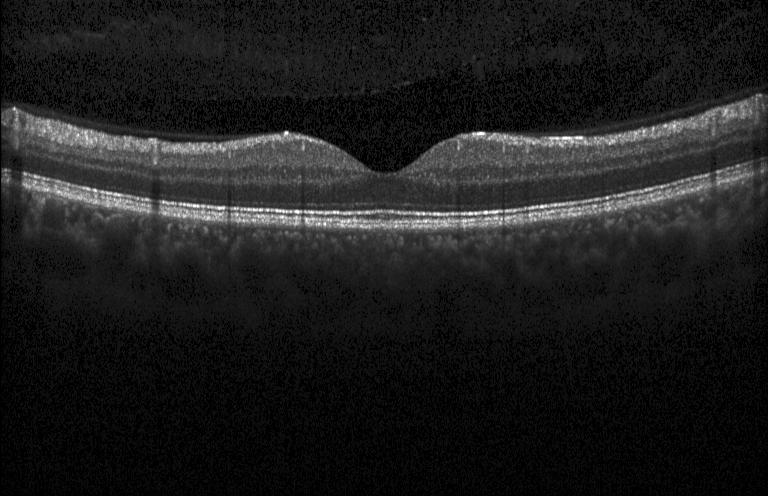

Acquired on a Heidelberg Spectralis. OCT B-scan — Impression: neither choroidal neovascularization, diabetic macular edema, nor drusen.